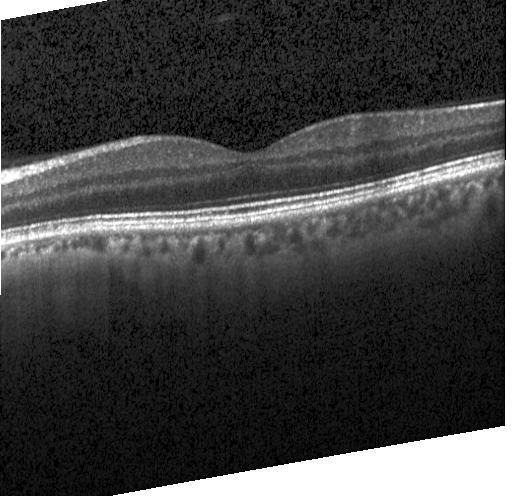

Retinal OCT cross-section.
Finding: no choroidal neovascularization, no diabetic macular edema, and no drusen.